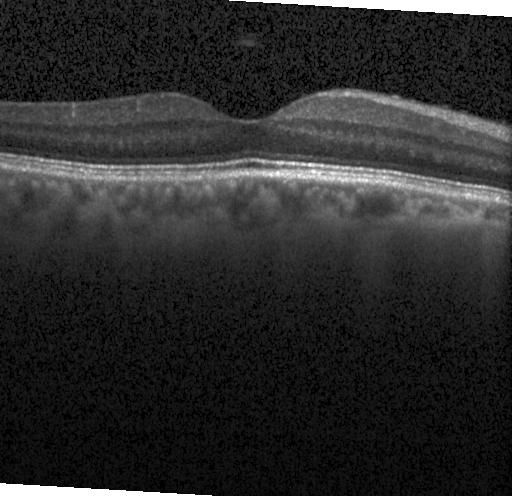 Retinal OCT B-scan; through the macula.
Finding: no evidence of choroidal neovascularization, diabetic macular edema, or drusen.